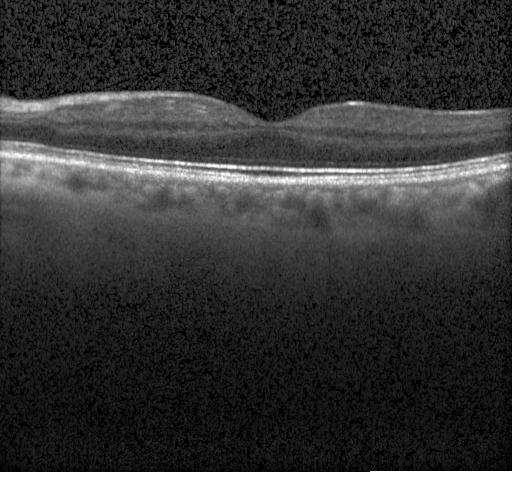
OCT scan showing no evidence of choroidal neovascularization, diabetic macular edema, or drusen.